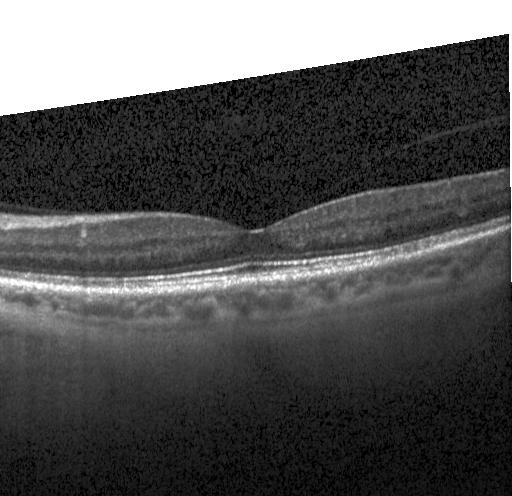
SD-OCT. Acquired on a Heidelberg Spectralis. Optical coherence tomography B-scan — Diagnosis: no evidence of choroidal neovascularization, diabetic macular edema, or drusen.